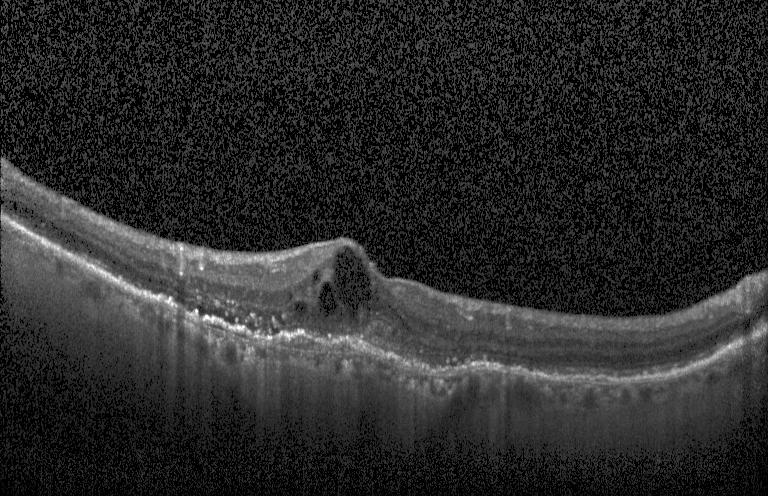
Retinal OCT B-scan, horizontal scan through the fovea, spectral-domain OCT, acquired on a Heidelberg Spectralis — Diagnosis: a choroidal neovascular membrane.